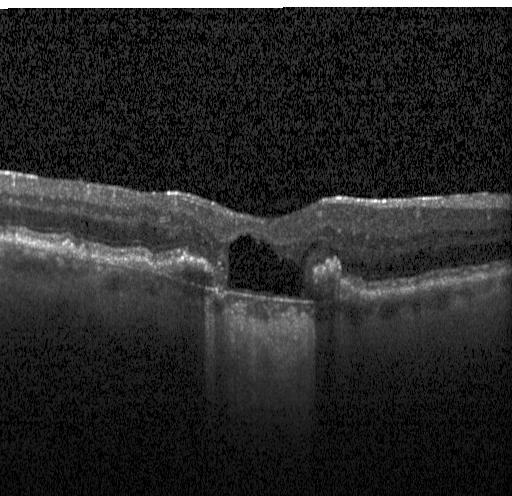
Finding: a choroidal neovascular membrane.